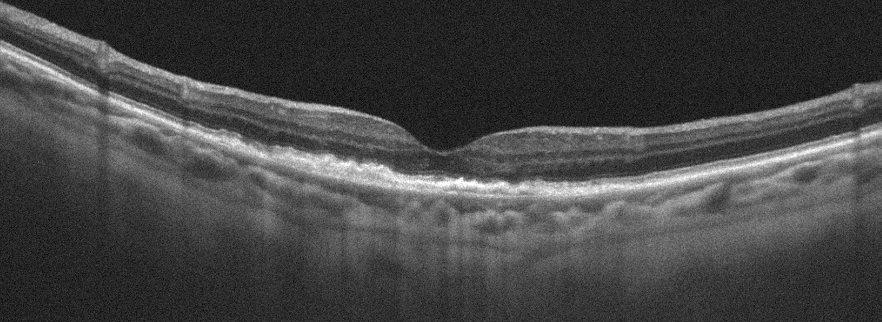 Through the macula, acquired on an Optovue Avanti RTVue XR, optical coherence tomography scan. AMD.